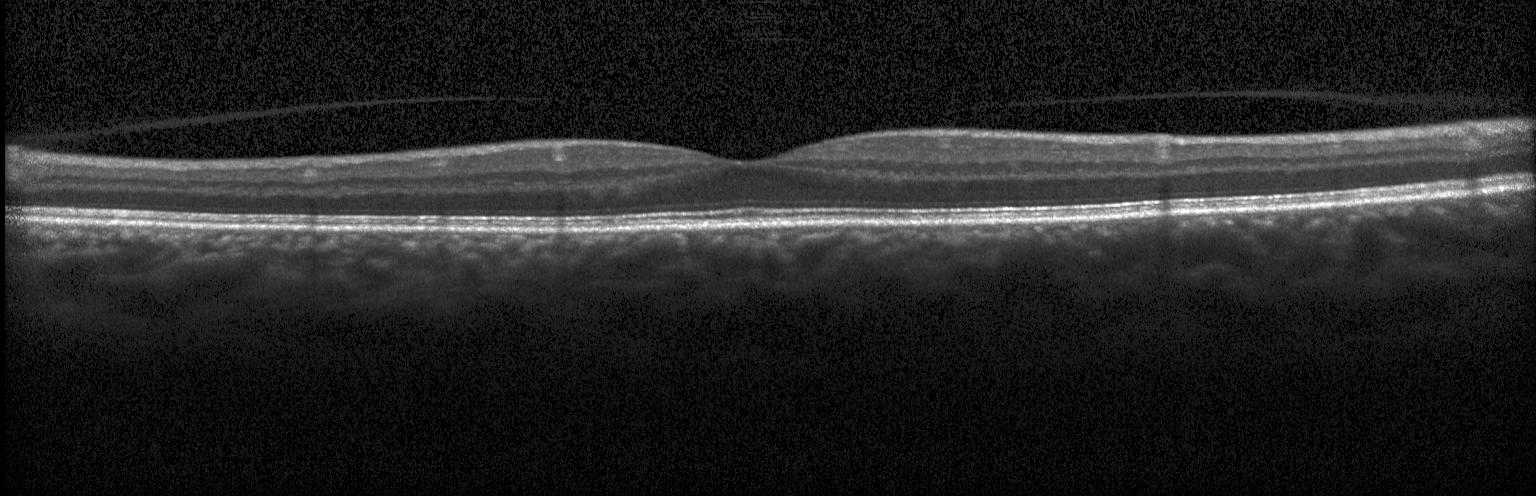
No choroidal neovascularization, diabetic macular edema, or drusen.